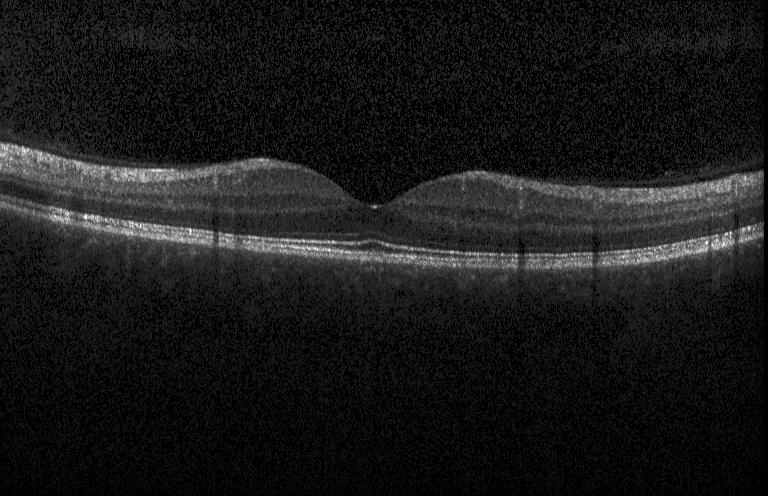

Dx: no evidence of choroidal neovascularization, diabetic macular edema, or drusen.